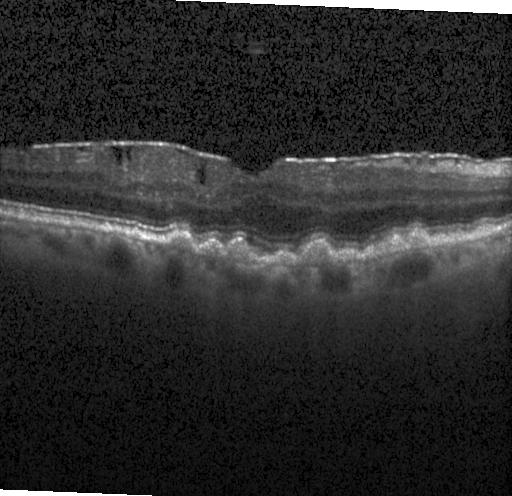

Retinal OCT B-scan.
Finding: sub-RPE drusenoid deposits.